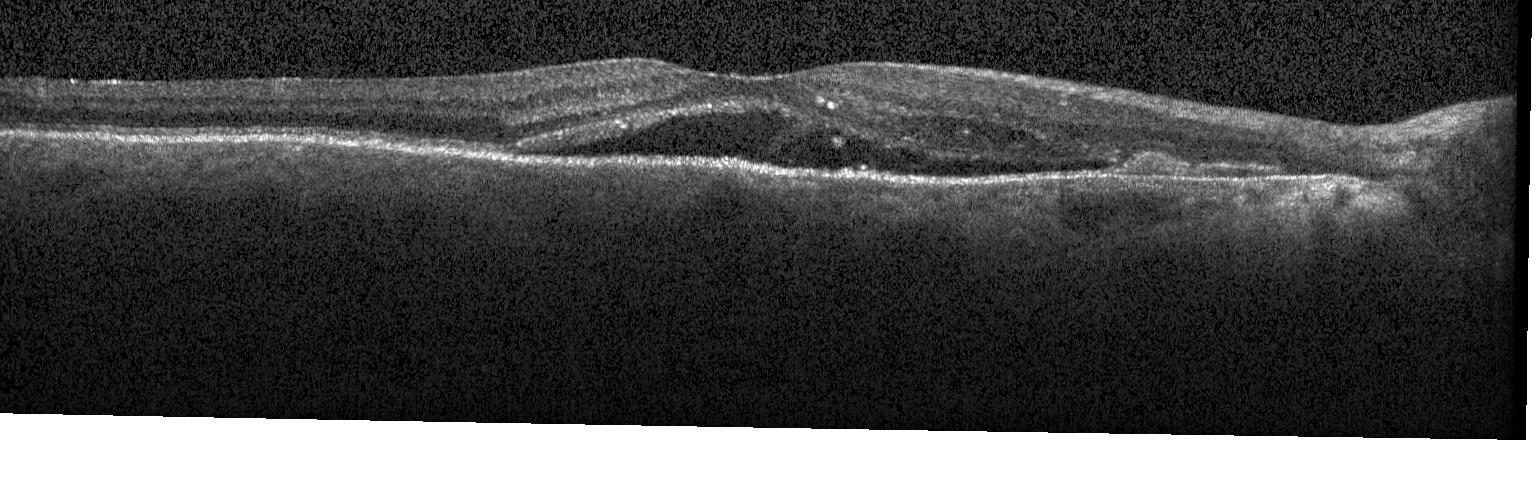

Spectral-domain OCT B-scan: CNV.